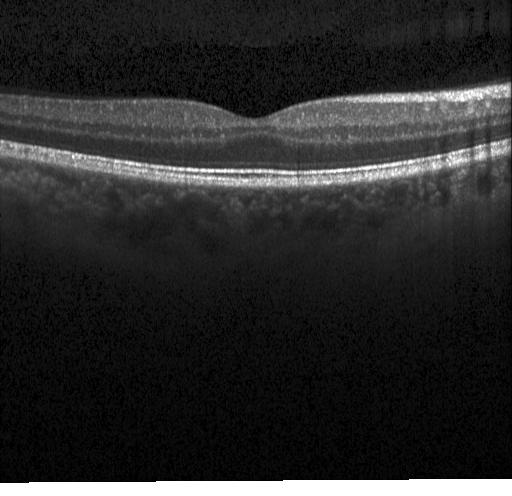
No choroidal neovascularization, no diabetic macular edema, and no drusen.